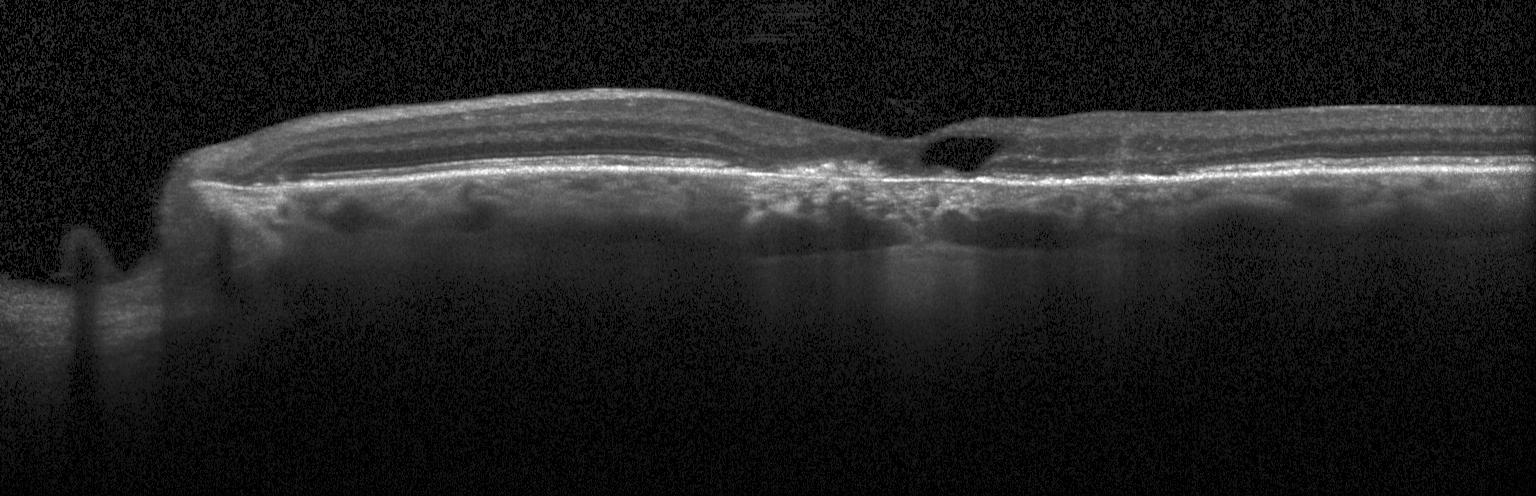
Macular OCT demonstrating a choroidal neovascular membrane.